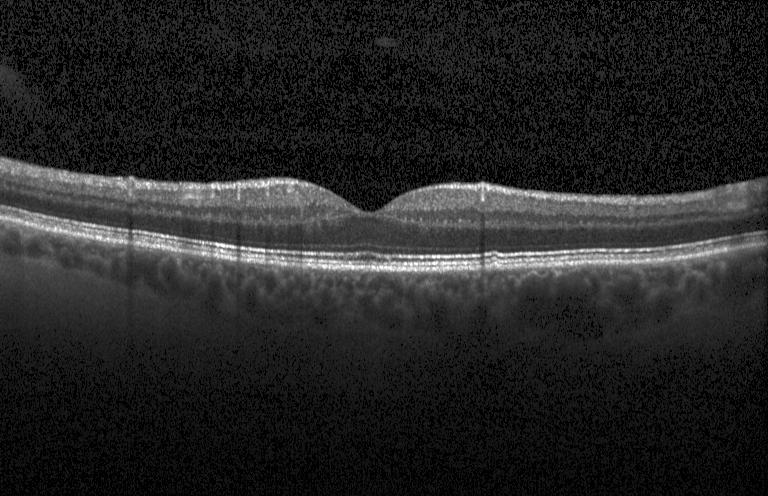 Centered on the fovea; OCT line scan
Diagnosis: neither choroidal neovascularization, diabetic macular edema, nor drusen.